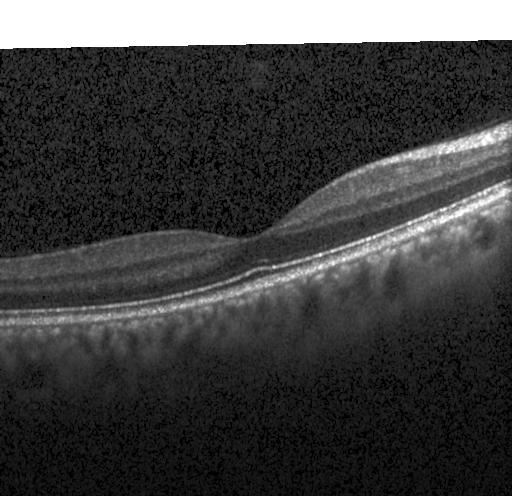

Dx: no evidence of CNV, DME, or drusen.